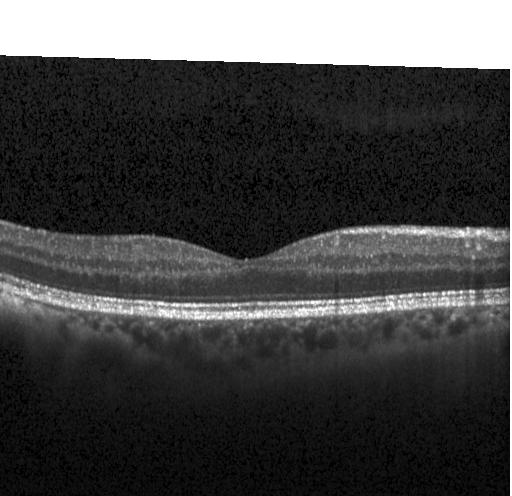
Finding: no CNV, DME, or drusen.